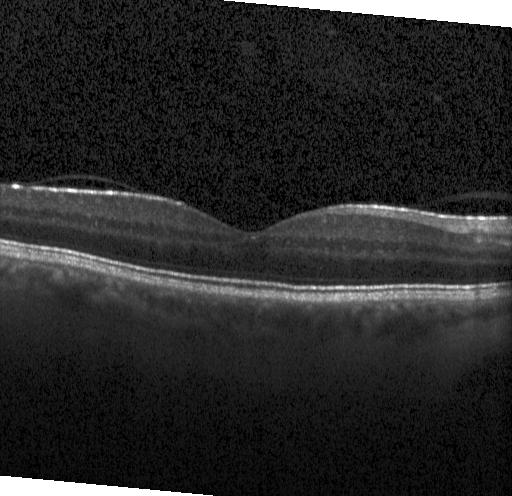 OCT B-scan. Diagnosis: no CNV, DME, or drusen.